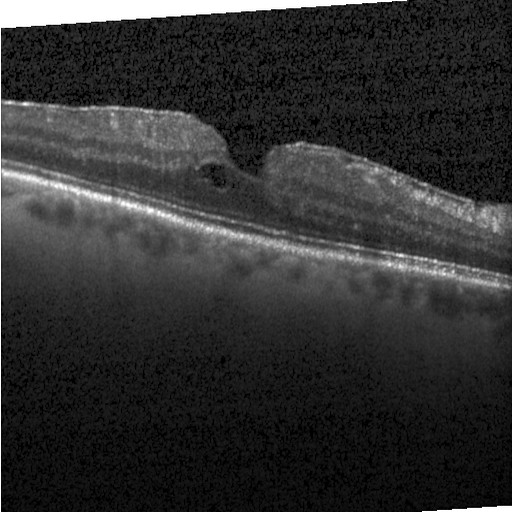 SD-OCT; OCT line scan; macular scan — Diagnosis: DME.